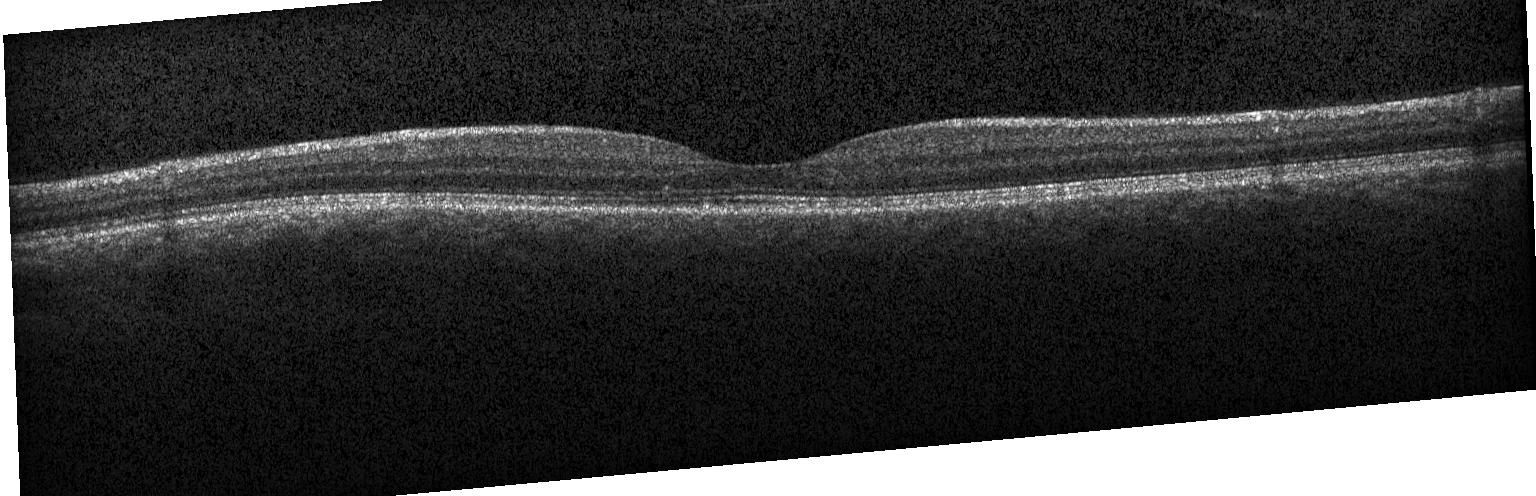

Macular OCT demonstrating no choroidal neovascularization, diabetic macular edema, or drusen.